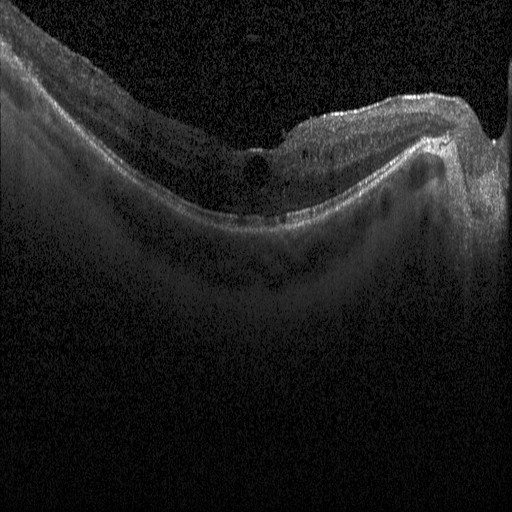
OCT line scan. Macular OCT: diabetic macular edema.